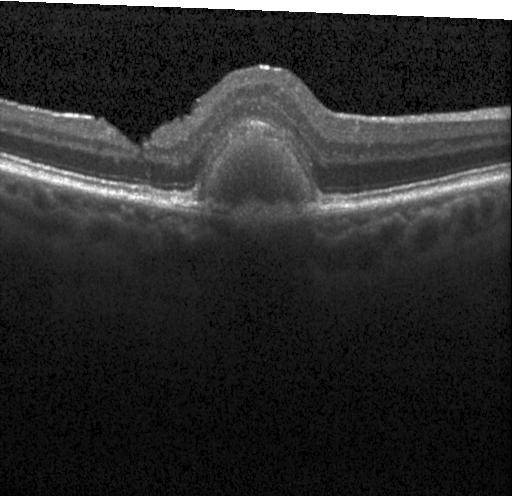 Optical coherence tomography B-scan
A choroidal neovascular membrane.